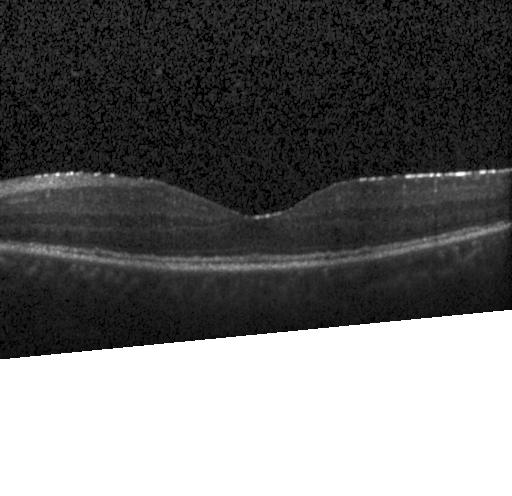

OCT B-scan showing no choroidal neovascularization, diabetic macular edema, or drusen.